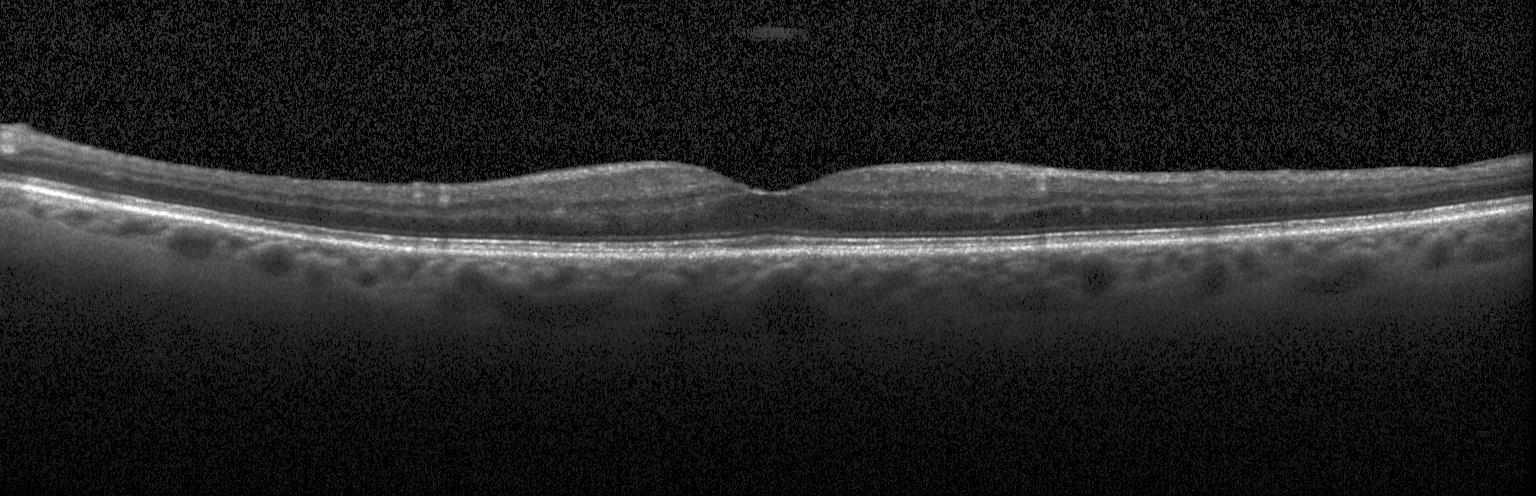

Macular OCT: no choroidal neovascularization, no diabetic macular edema, and no drusen.